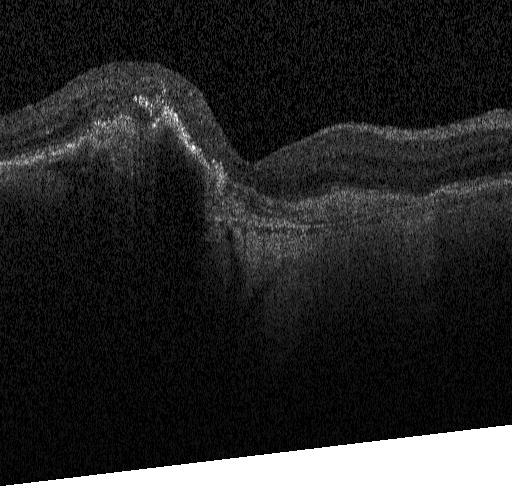
Optical coherence tomography B-scan · spectral-domain optical coherence tomography. Finding: a choroidal neovascular membrane.